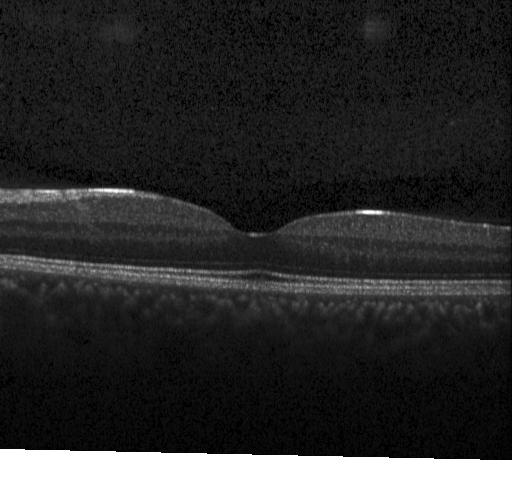
Retinal OCT B-scan, Heidelberg Spectralis OCT system, fovea-centered — Finding: neither choroidal neovascularization, diabetic macular edema, nor drusen.